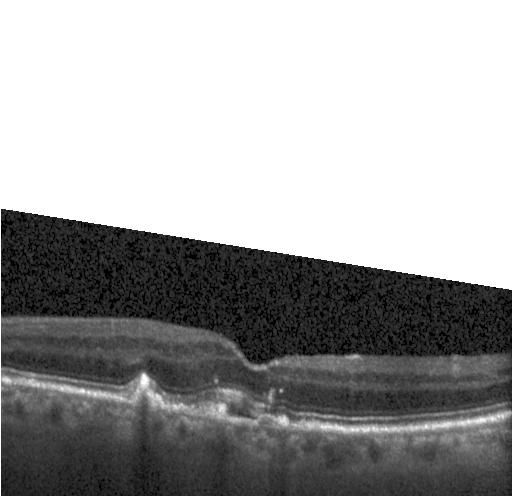

Retinal OCT cross-section
Impression: CNV.